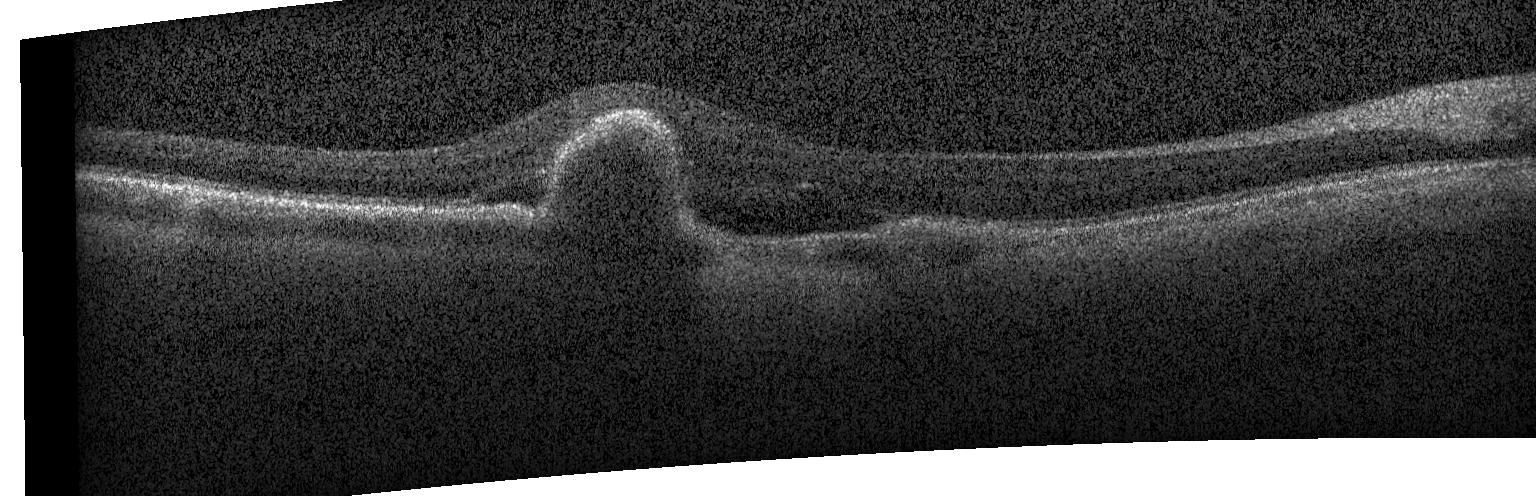
A choroidal neovascular membrane.